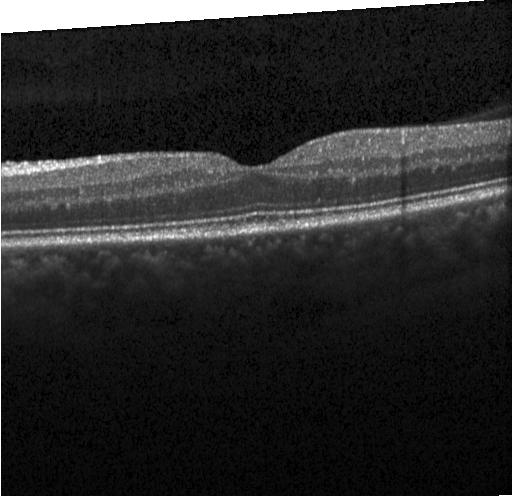
Dx: no choroidal neovascularization, no diabetic macular edema, and no drusen.